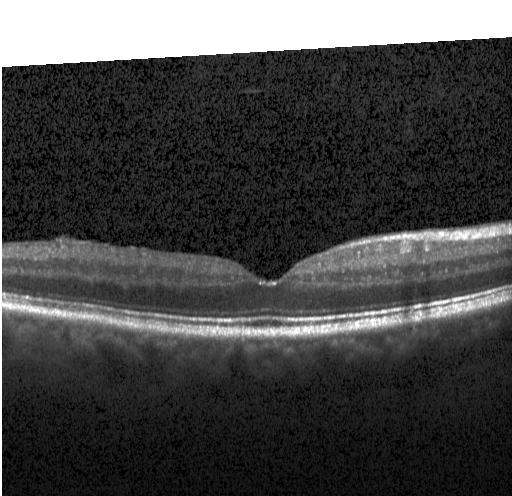
OCT line scan. Macular OCT: no CNV, DME, or drusen.